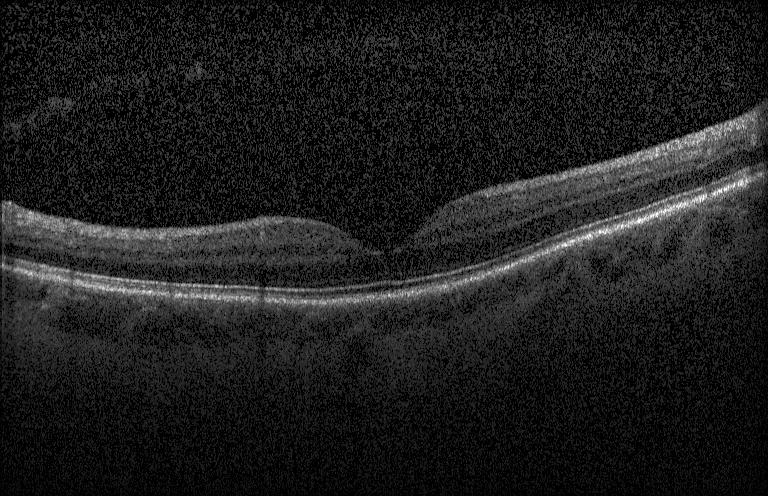

No CNV, DME, or drusen.